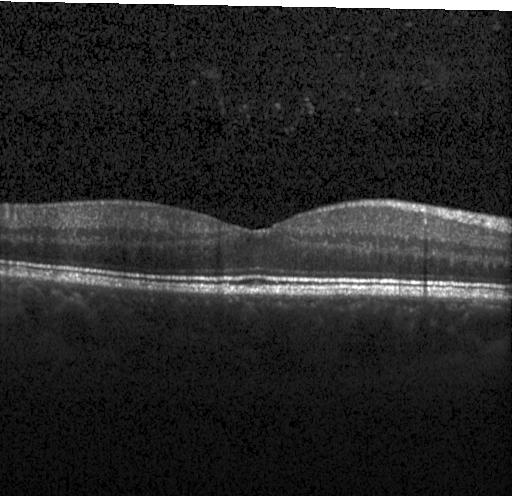

Through the macula. Heidelberg Spectralis OCT system. SD-OCT. Retinal OCT B-scan
Assessment: no CNV, DME, or drusen.